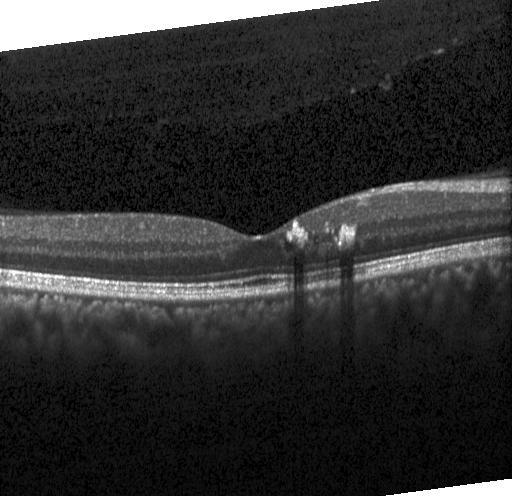

OCT B-scan. Centered on the fovea. SD-OCT — OCT finding: neither choroidal neovascularization, diabetic macular edema, nor drusen.